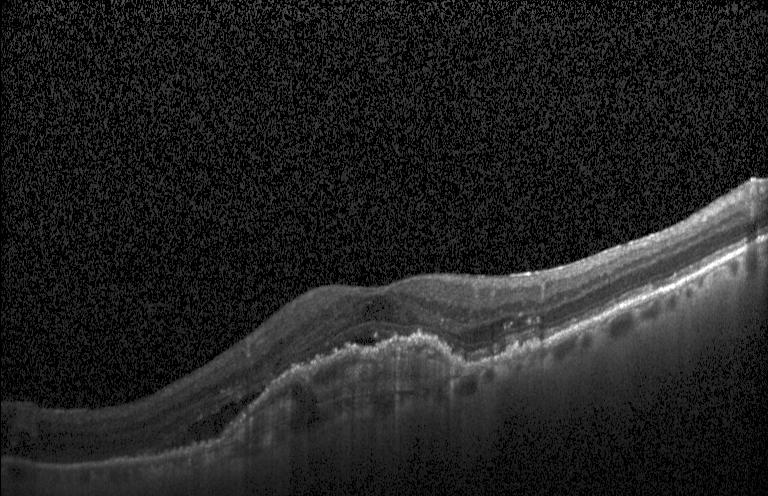 Impression: a choroidal neovascular membrane.